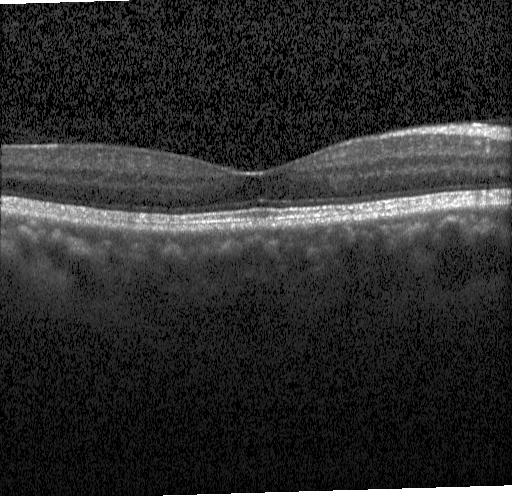

Retinal OCT B-scan
Diagnosis: no choroidal neovascularization, no diabetic macular edema, and no drusen.